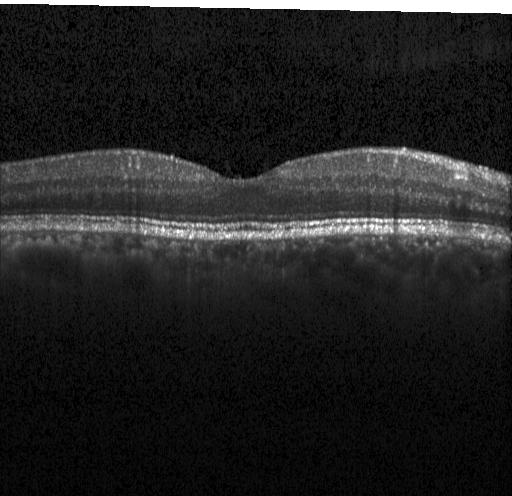 Retinal OCT B-scan. Finding: no evidence of choroidal neovascularization, diabetic macular edema, or drusen.